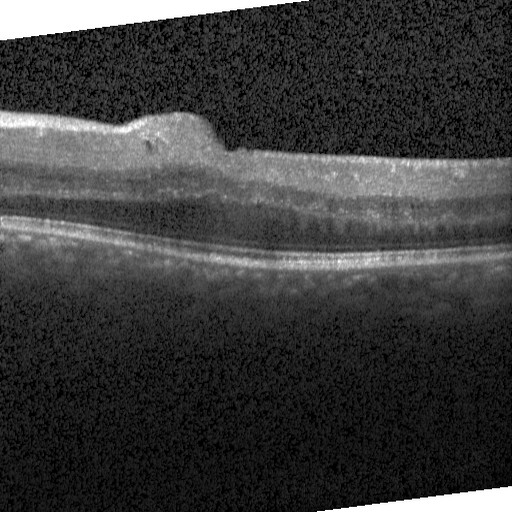

OCT finding: DME.